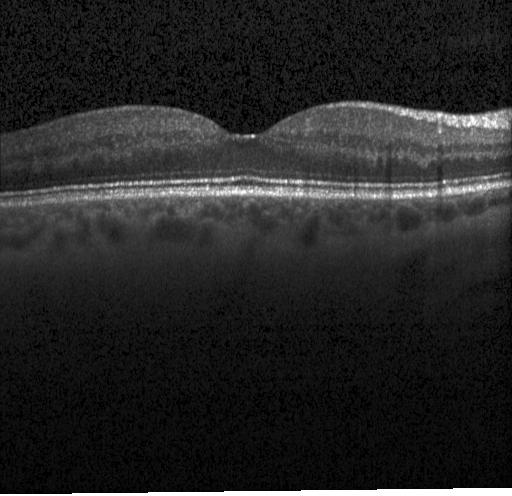
The scan shows neither CNV, DME, nor drusen.